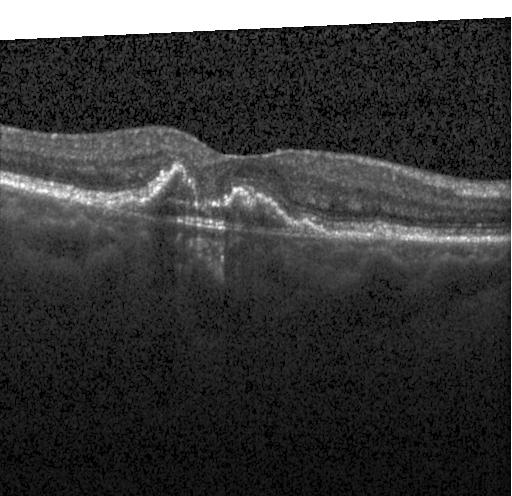
Macular scan, acquired on a Heidelberg Spectralis, OCT line scan, spectral-domain optical coherence tomography.
The scan shows choroidal neovascularization.